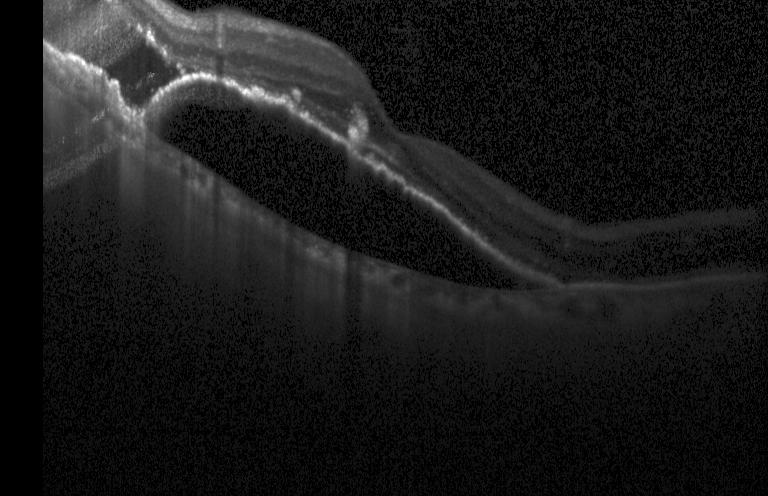
Through the macula. OCT B-scan. Assessment: CNV.